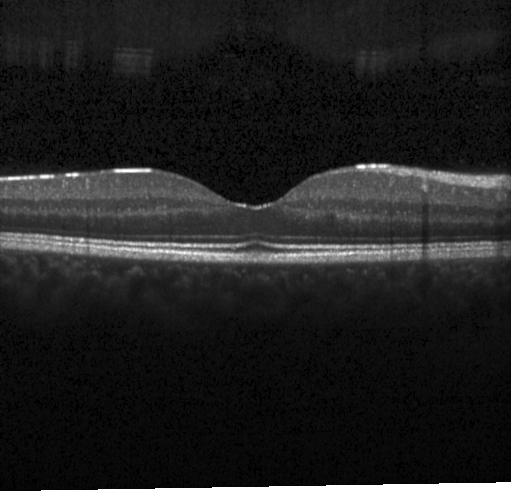 OCT line scan. SD-OCT. Horizontal scan through the fovea — The scan shows no choroidal neovascularization, no diabetic macular edema, and no drusen.